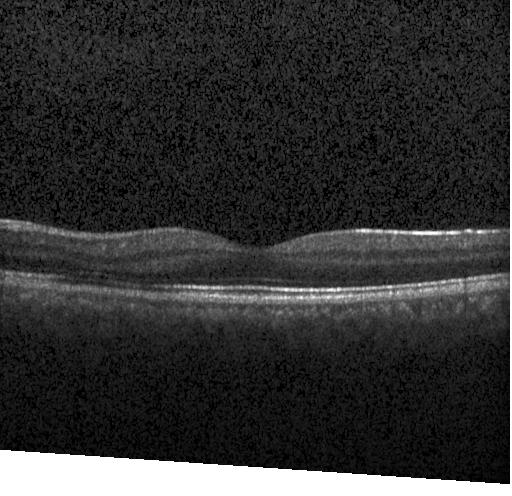

Fovea-centered · OCT line scan.
Finding: no choroidal neovascularization, diabetic macular edema, or drusen.